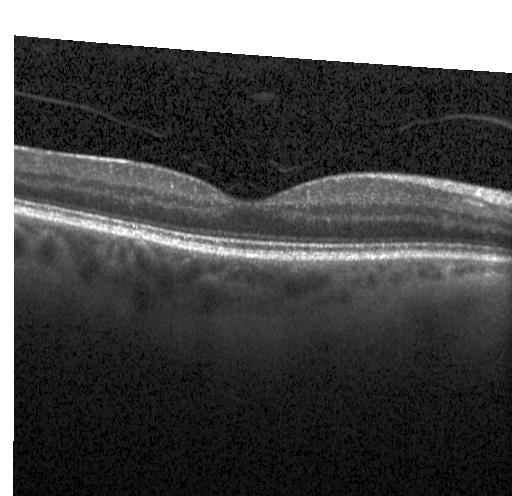

Retinal OCT B-scan
Assessment: no CNV, no DME, and no drusen.